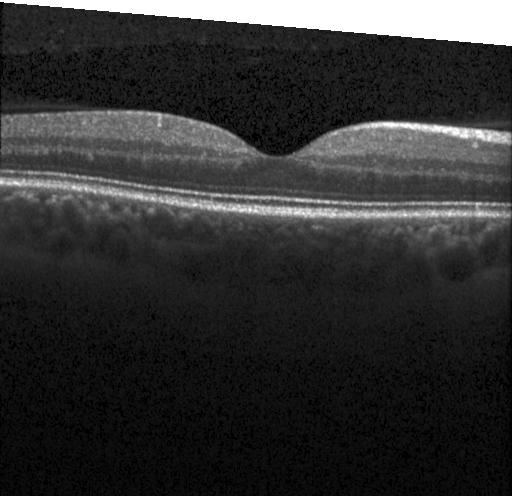

Instrument: Heidelberg Spectralis; OCT line scan; SD-OCT; through the macula
This B-scan demonstrates no choroidal neovascularization, diabetic macular edema, or drusen.